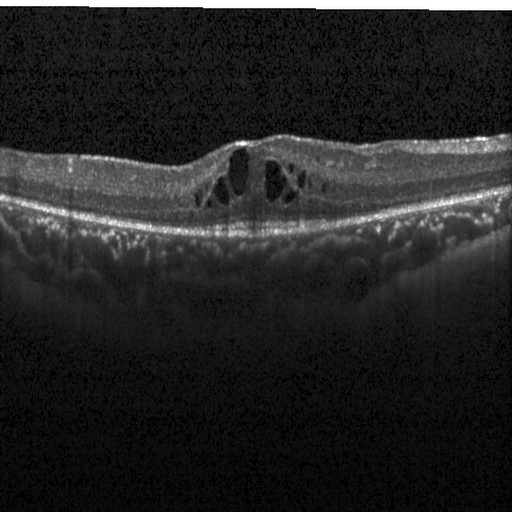 Retinal OCT B-scan; spectral-domain optical coherence tomography; Heidelberg Spectralis OCT system. OCT finding: diabetic macular edema.